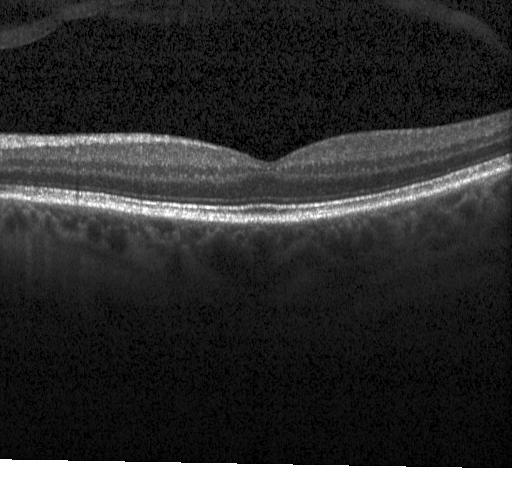
OCT B-scan · instrument: Heidelberg Spectralis · fovea-centered.
Macular OCT: neither choroidal neovascularization, diabetic macular edema, nor drusen.